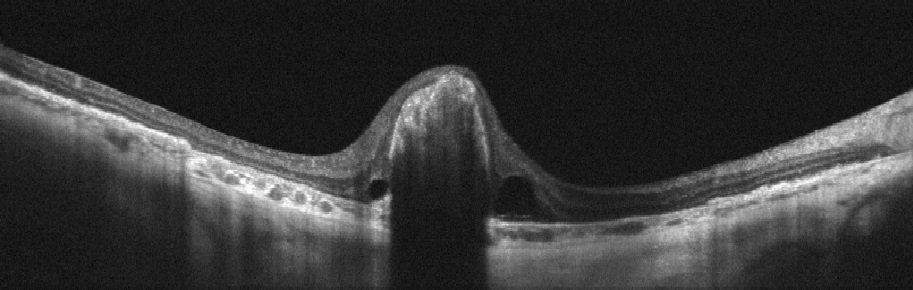 Optical coherence tomography B-scan.
Impression: AMD.